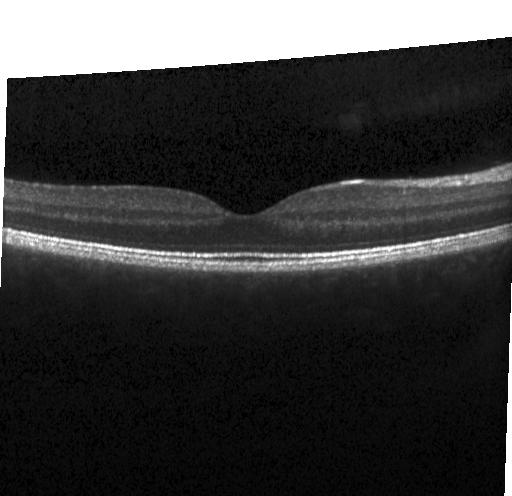

Impression: no evidence of CNV, DME, or drusen.